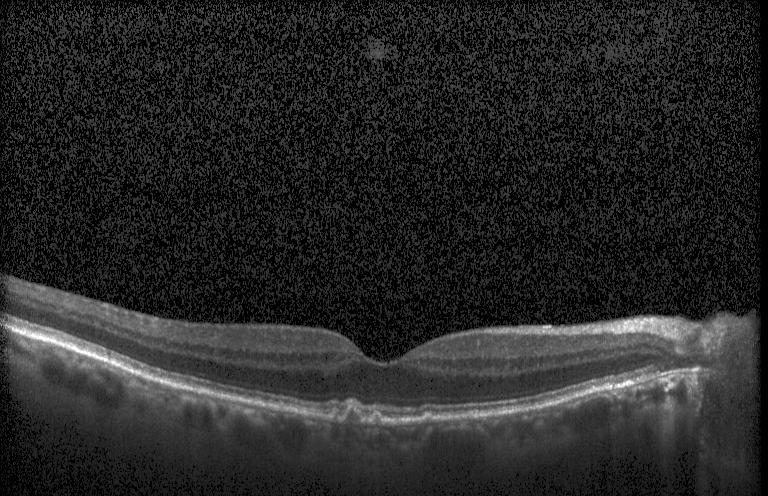 Macular OCT demonstrating multiple drusen.